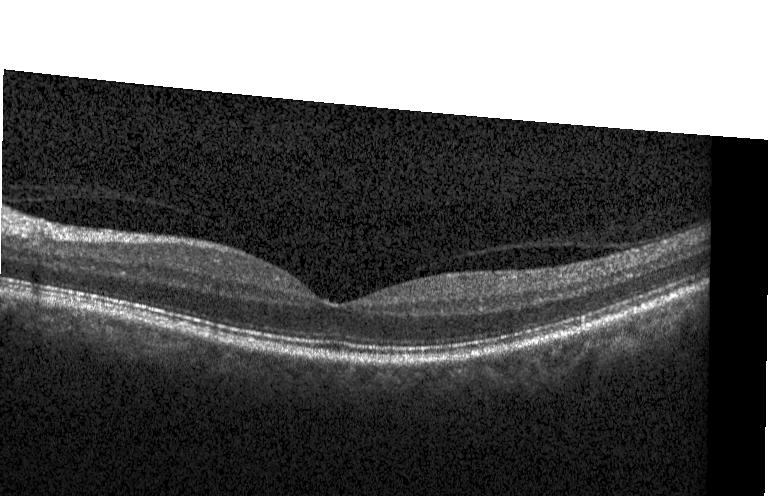
Spectral-domain OCT; macular scan; retinal OCT B-scan; Heidelberg Spectralis
This B-scan demonstrates no choroidal neovascularization, diabetic macular edema, or drusen.